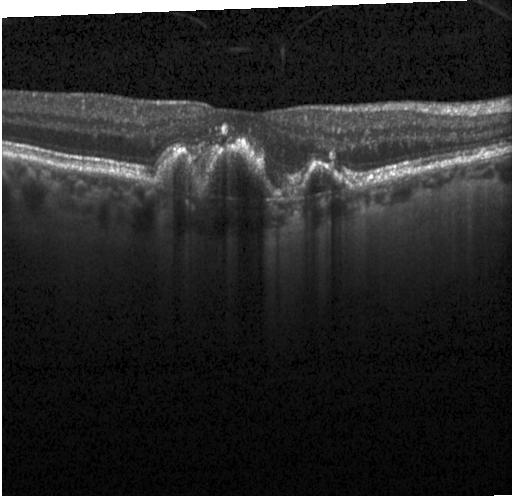 OCT B-scan — Diagnosis: choroidal neovascularization.